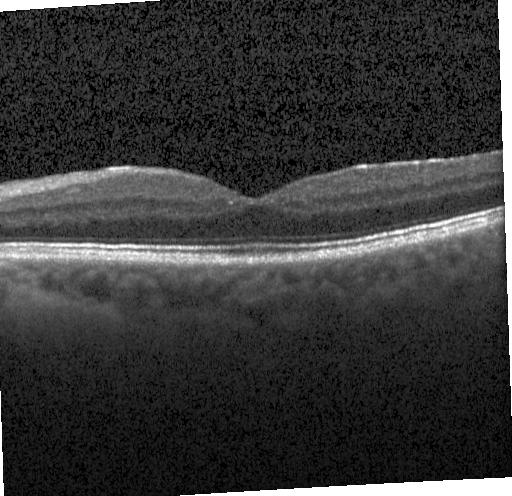
Spectral-domain OCT B-scan: no CNV, no DME, and no drusen.